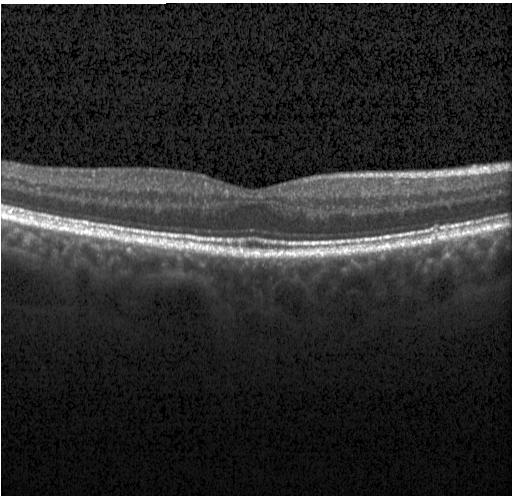 Instrument: Heidelberg Spectralis; retinal OCT cross-section. OCT finding: no evidence of CNV, DME, or drusen.